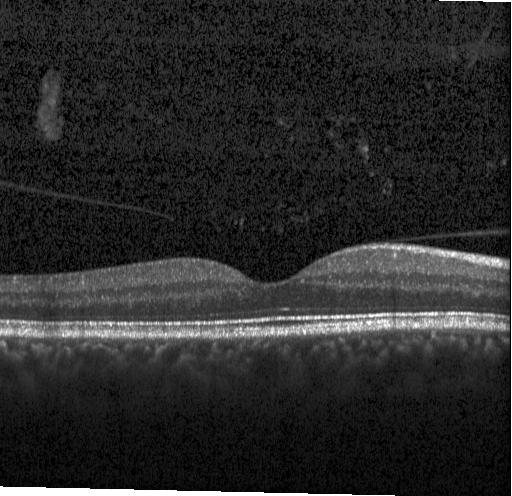

OCT B-scan showing no CNV, no DME, and no drusen.